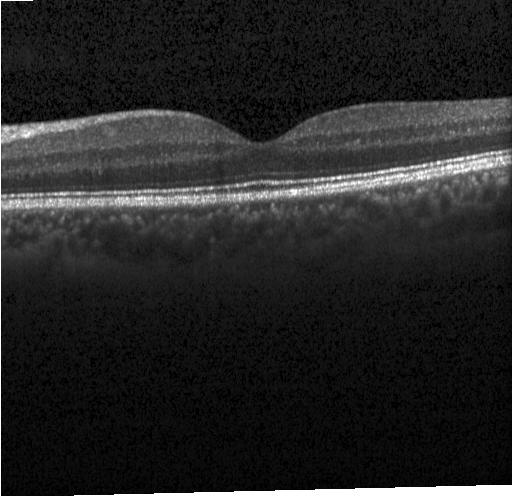

Macular scan, acquired on a Heidelberg Spectralis, spectral-domain OCT, OCT B-scan.
Impression: neither CNV, DME, nor drusen.